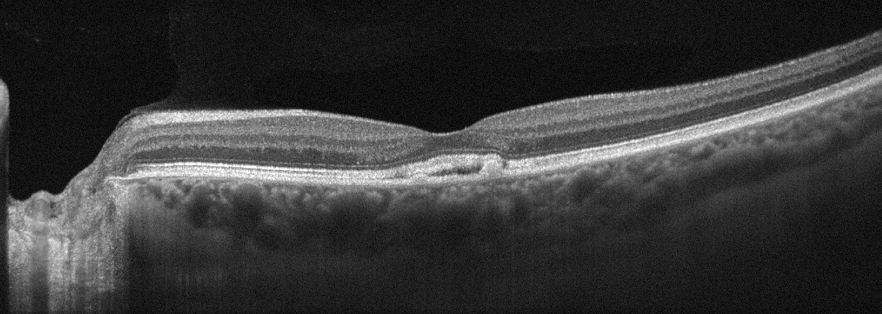 OS; optical coherence tomography scan. Assessment: AMD.